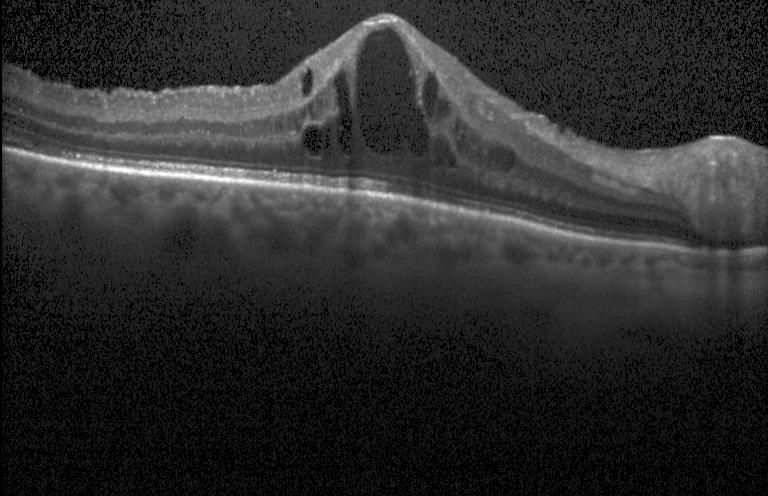
Retinal OCT cross-section showing DME.